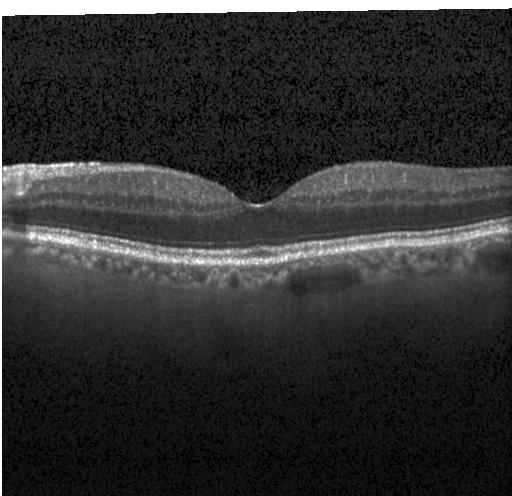 No evidence of choroidal neovascularization, diabetic macular edema, or drusen.